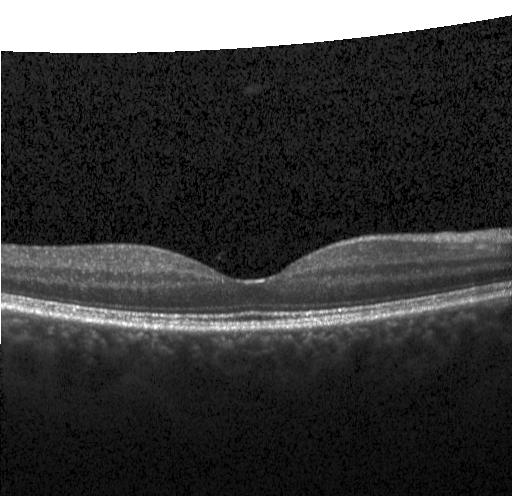 OCT B-scan. Macular OCT: no choroidal neovascularization, no diabetic macular edema, and no drusen.